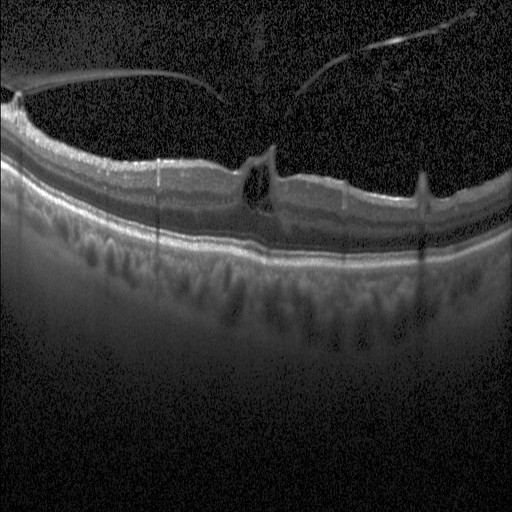
Optical coherence tomography B-scan — Finding: diabetic macular edema (DME).